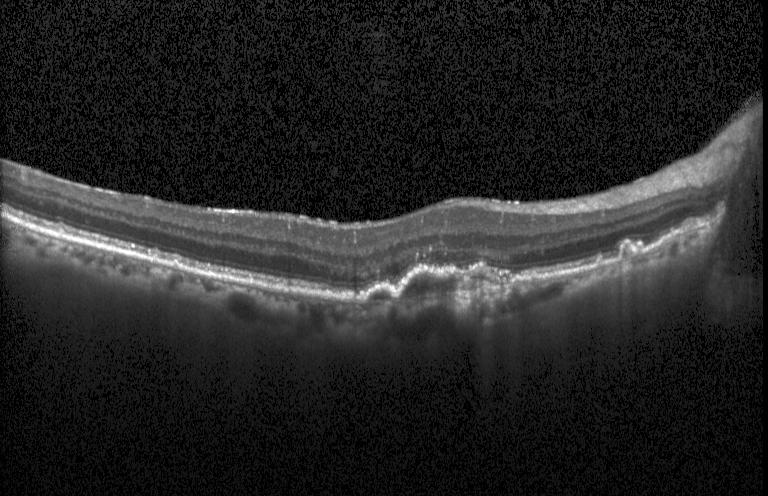
OCT B-scan showing choroidal neovascularization (CNV).